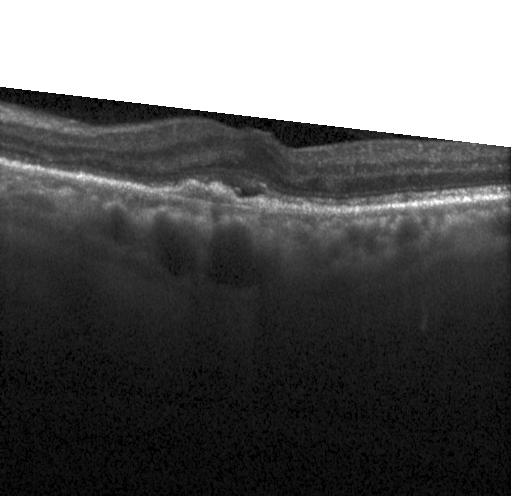
Retinal OCT cross-section showing choroidal neovascularization (CNV).